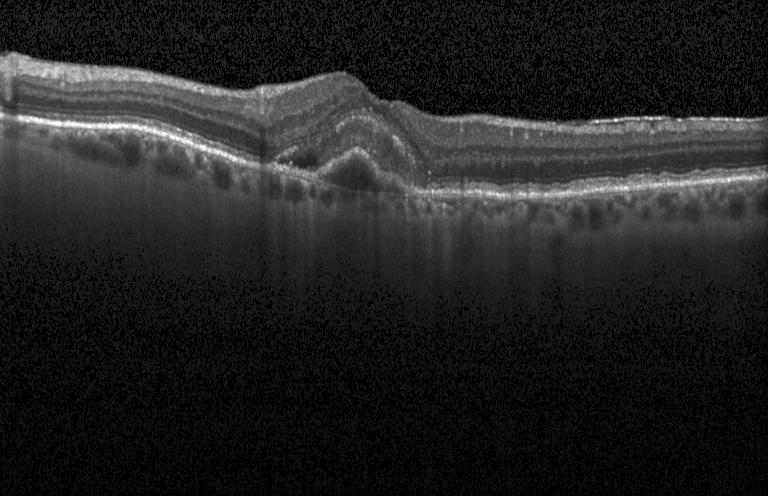

Spectral-domain optical coherence tomography. OCT B-scan — Dx: choroidal neovascularization.